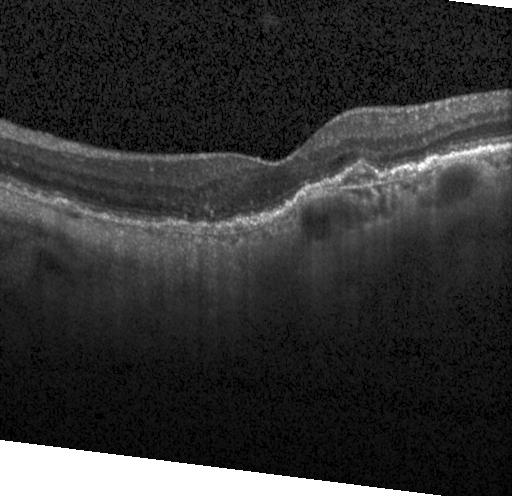 Spectral-domain optical coherence tomography · retinal OCT cross-section · Heidelberg Spectralis OCT system · horizontal scan through the fovea.
Finding: a choroidal neovascular membrane.